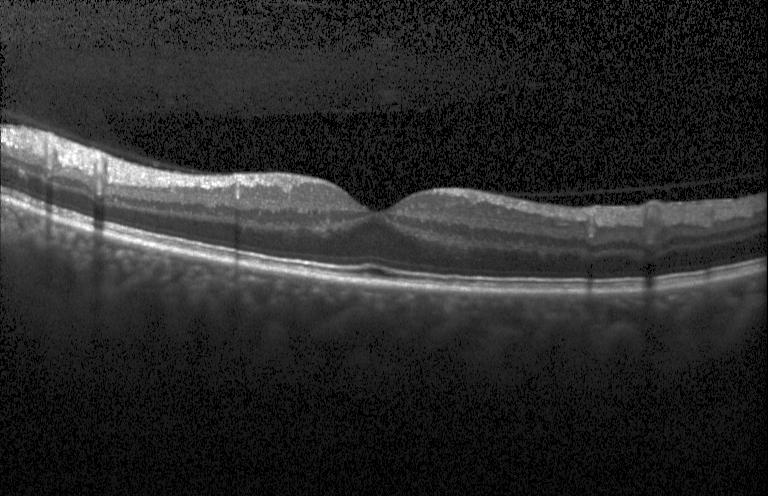
Retinal OCT B-scan. OCT finding: no choroidal neovascularization, diabetic macular edema, or drusen.